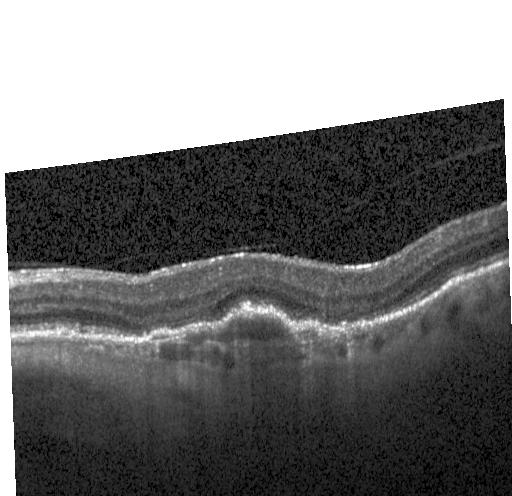 CNV.